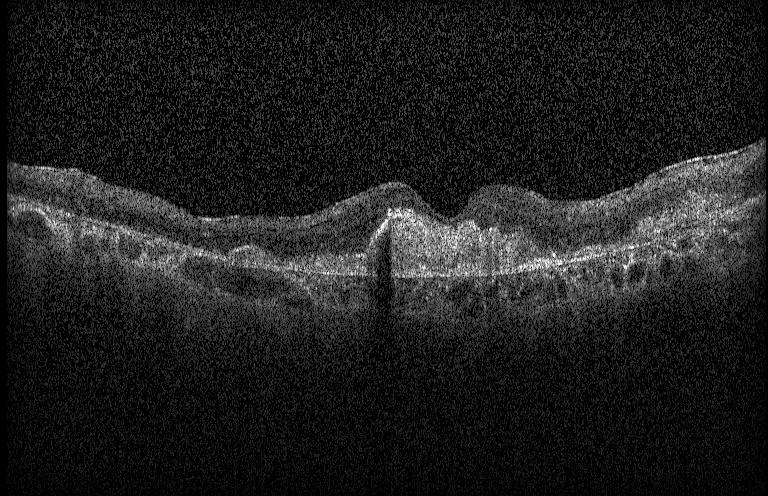
OCT B-scan — Finding: a choroidal neovascular membrane.